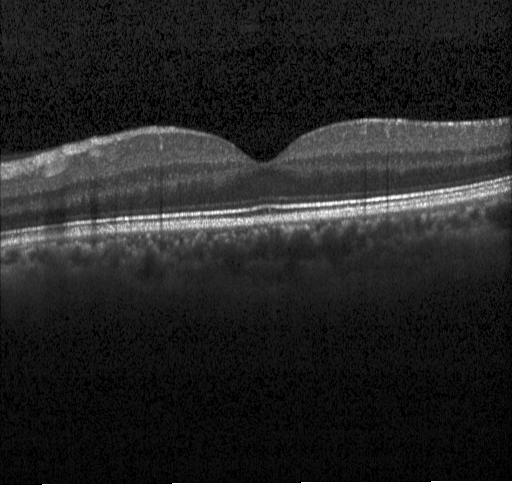 Spectral-domain OCT B-scan: neither CNV, DME, nor drusen.